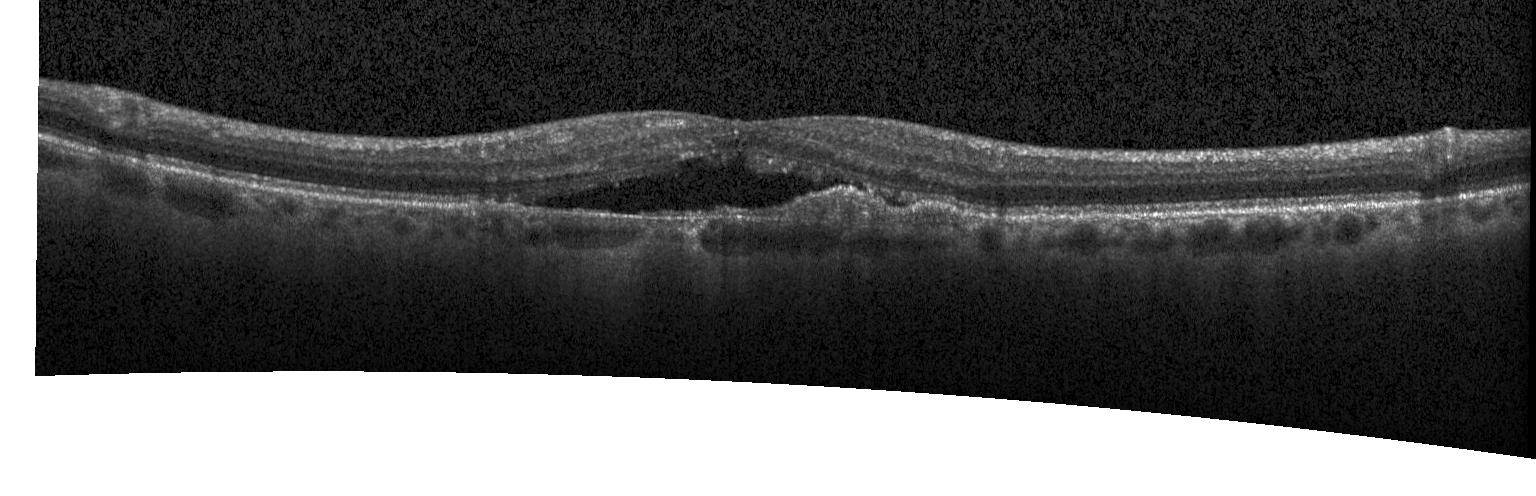

OCT line scan — This B-scan demonstrates a choroidal neovascular membrane.